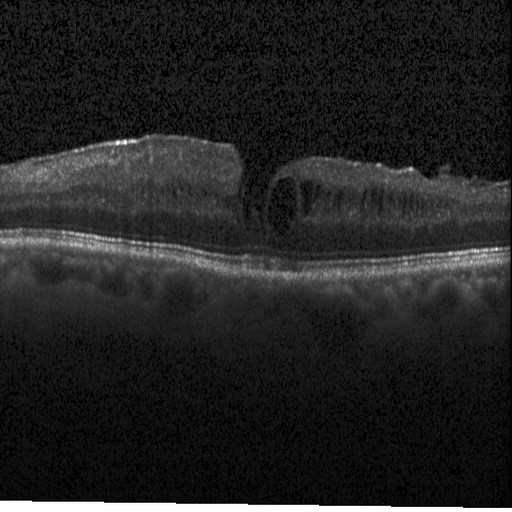

Diagnosis: diabetic macular edema (DME).